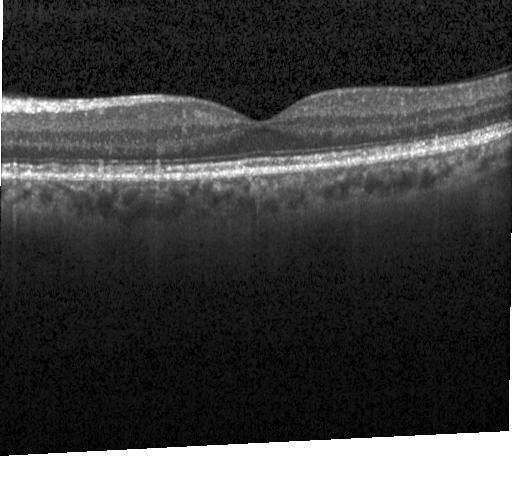 Retinal OCT cross-section; SD-OCT.
Dx: no choroidal neovascularization, diabetic macular edema, or drusen.